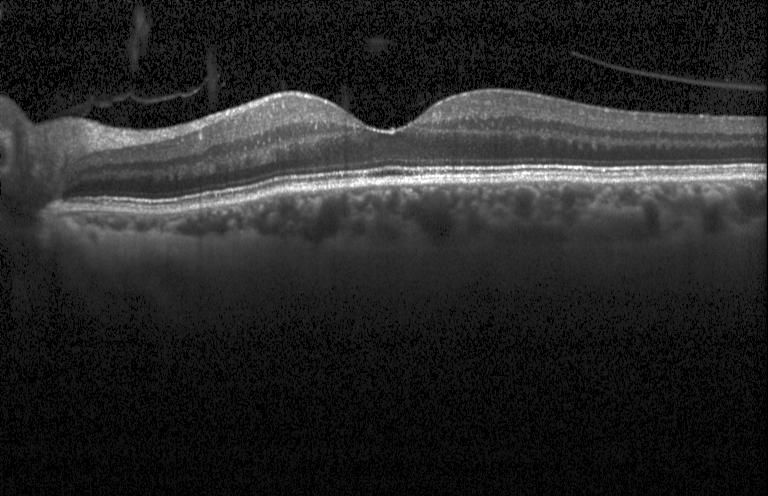

SD-OCT · optical coherence tomography B-scan
No choroidal neovascularization, diabetic macular edema, or drusen.